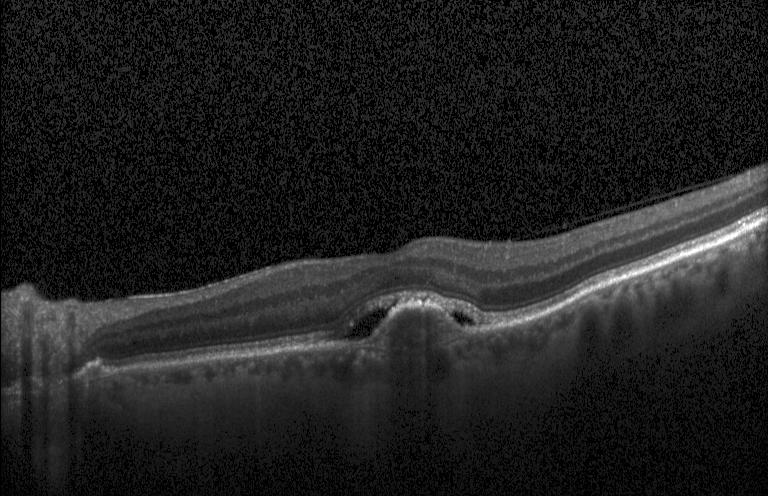

Centered on the fovea. Optical coherence tomography scan. Spectral-domain optical coherence tomography.
Choroidal neovascularization (CNV).